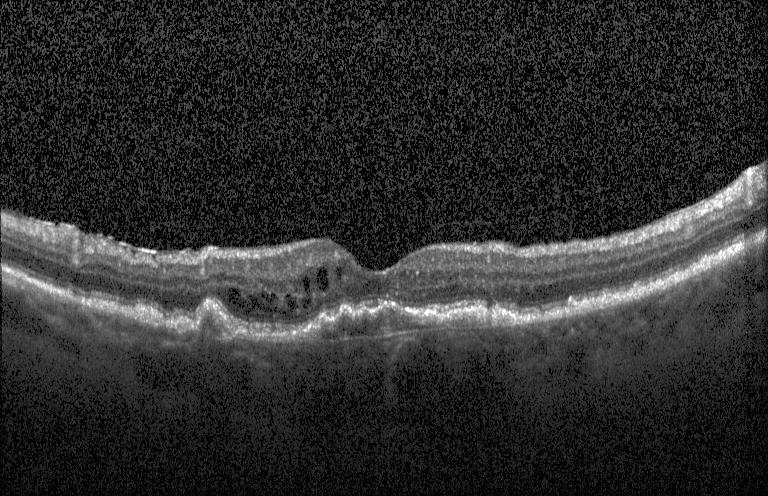 Optical coherence tomography B-scan; Heidelberg Spectralis.
Finding: choroidal neovascularization.